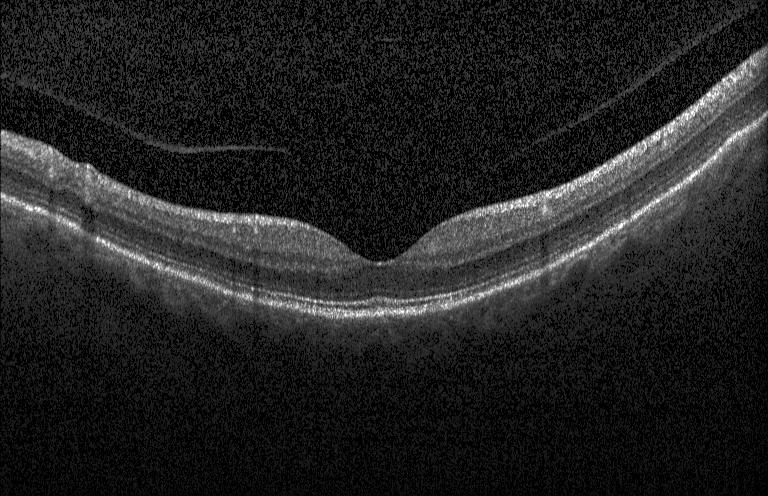
OCT finding: no evidence of choroidal neovascularization, diabetic macular edema, or drusen.